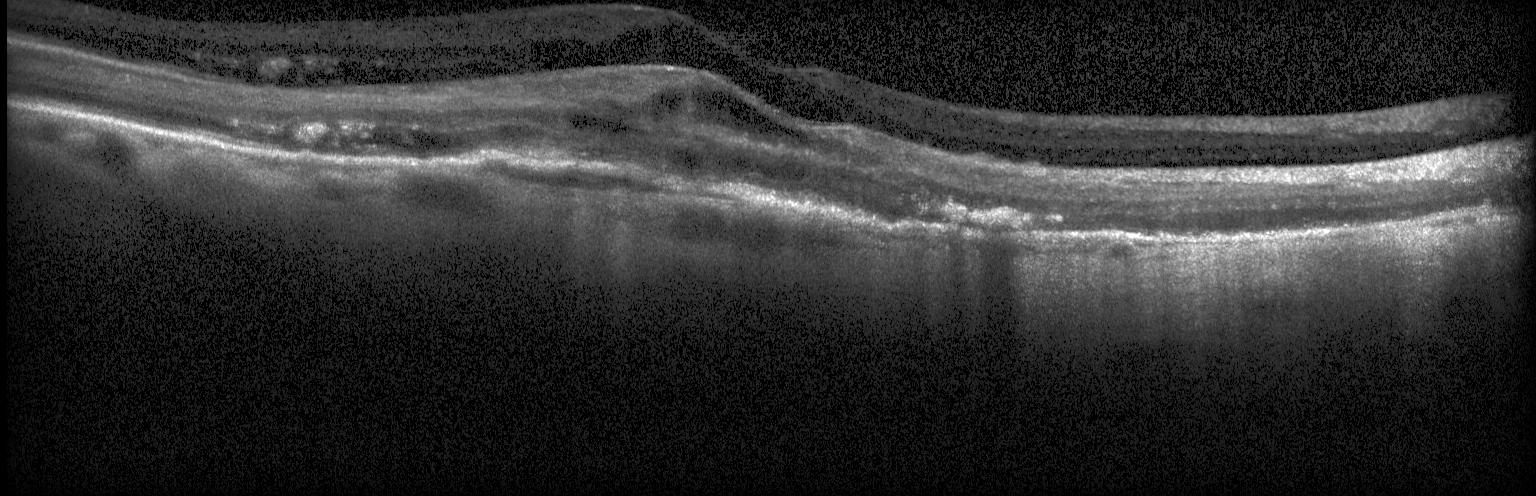

Impression: choroidal neovascularization.